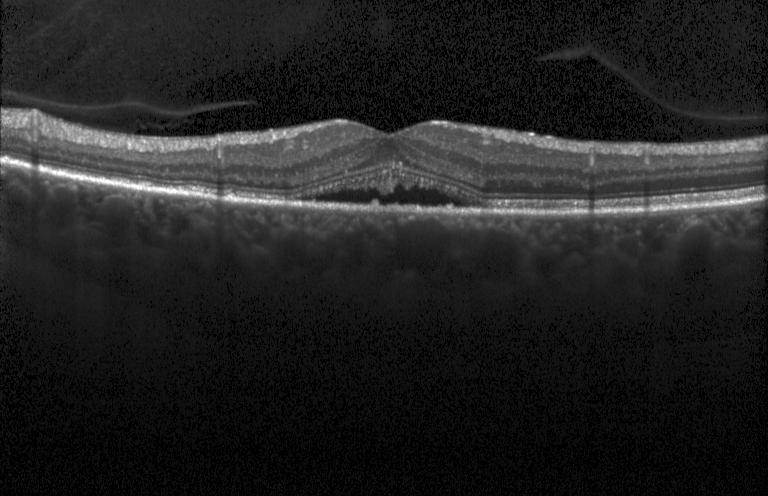
Heidelberg Spectralis. Spectral-domain OCT. Retinal OCT B-scan
Assessment: a choroidal neovascular membrane.